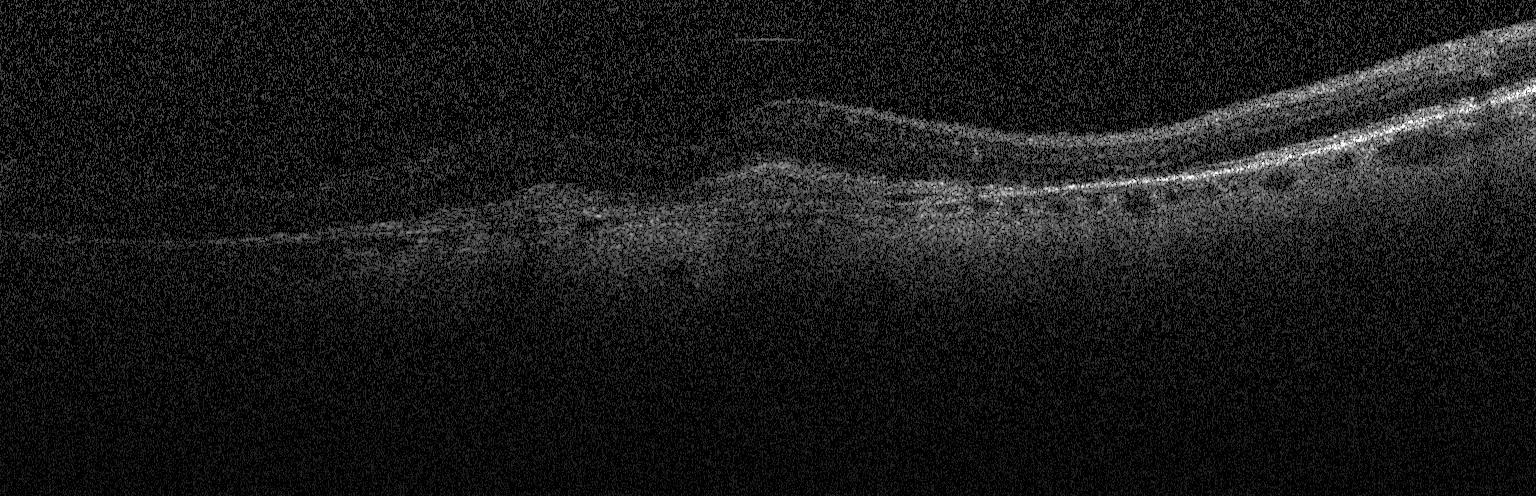
SD-OCT · OCT B-scan · horizontal scan through the fovea · acquired on a Heidelberg Spectralis. Dx: choroidal neovascularization (CNV).